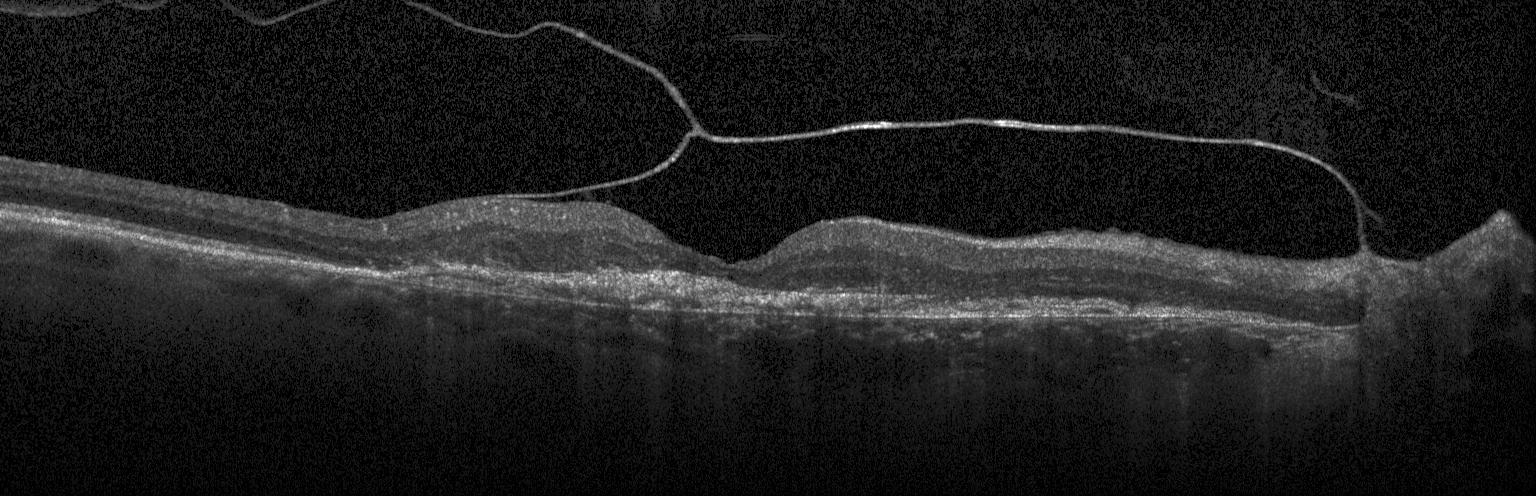
OCT B-scan
Diagnosis: choroidal neovascularization.